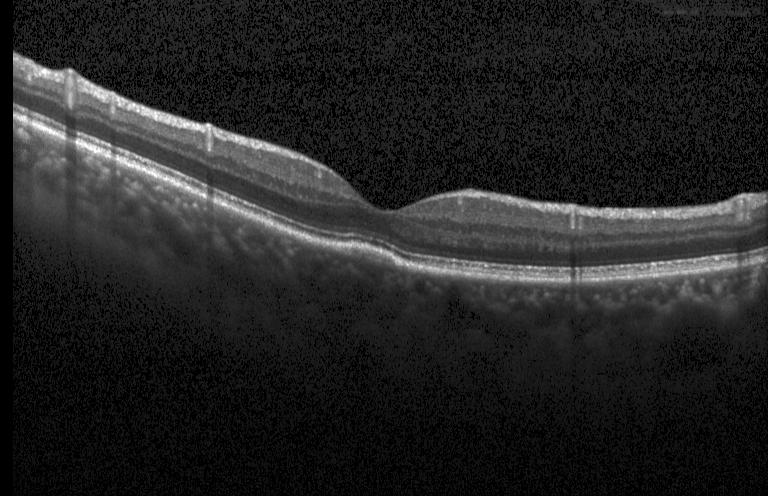 Optical coherence tomography B-scan. Diagnosis: multiple drusen.